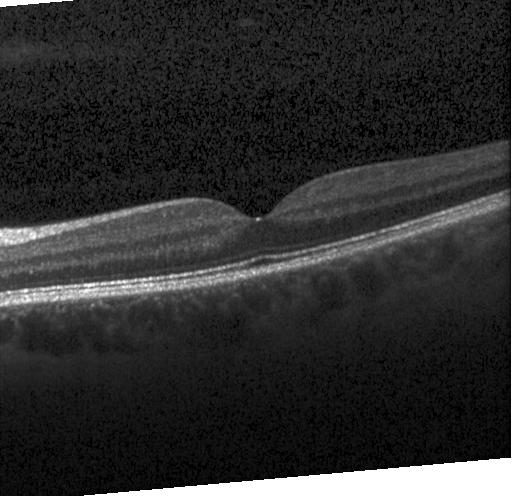
Heidelberg Spectralis · spectral-domain optical coherence tomography · macular scan · retinal OCT cross-section. OCT finding: no evidence of choroidal neovascularization, diabetic macular edema, or drusen.